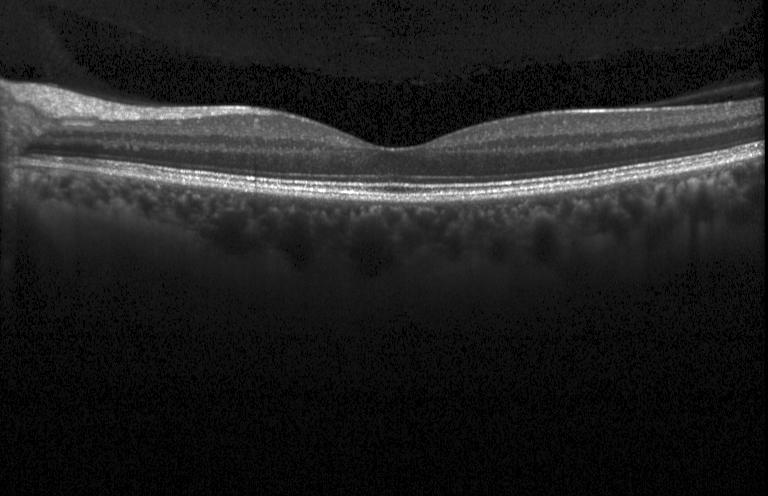

Finding: no choroidal neovascularization, no diabetic macular edema, and no drusen.